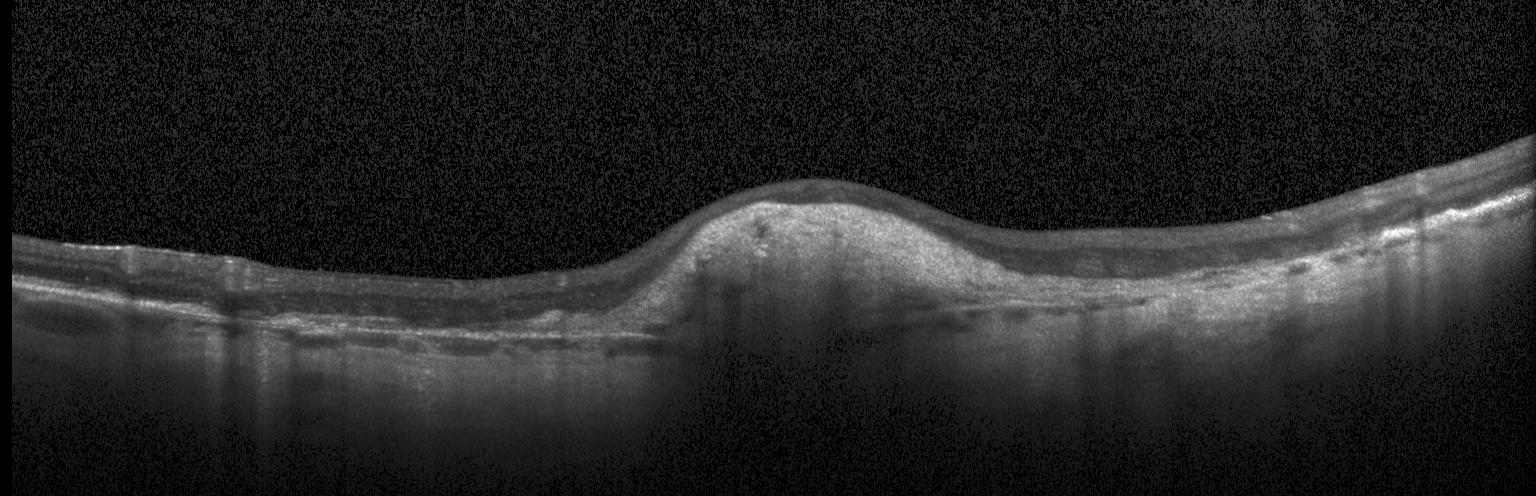 Spectral-domain OCT B-scan: choroidal neovascularization (CNV).